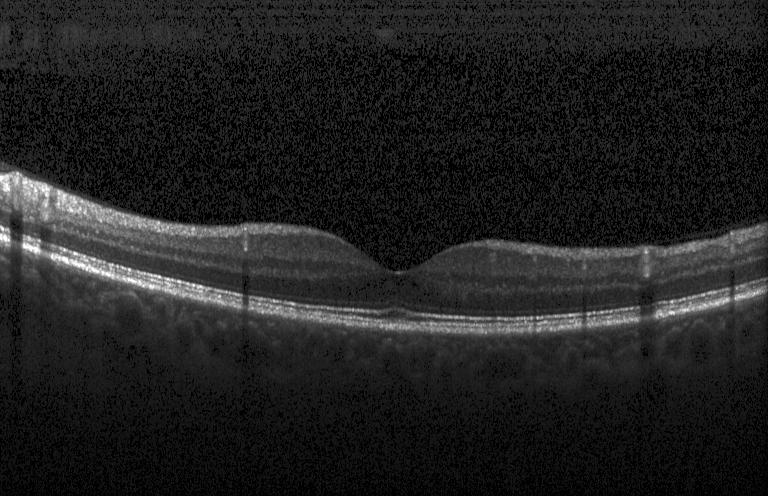 This B-scan demonstrates neither CNV, DME, nor drusen.